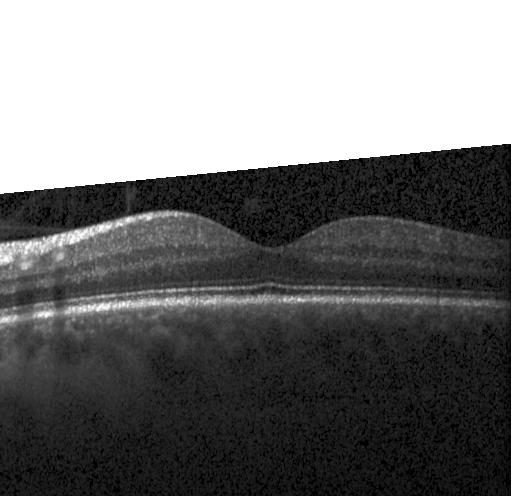 Diagnosis: no CNV, DME, or drusen.